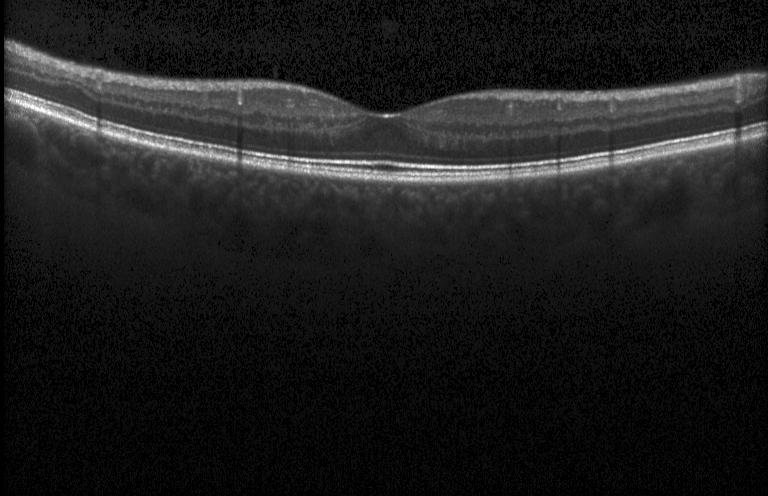
OCT line scan — Assessment: no evidence of CNV, DME, or drusen.